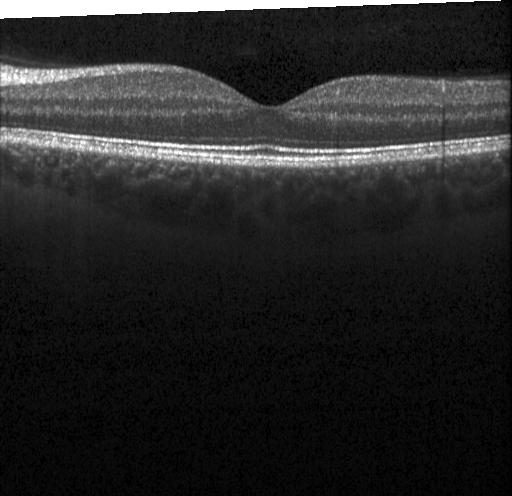
Finding: no choroidal neovascularization, diabetic macular edema, or drusen.